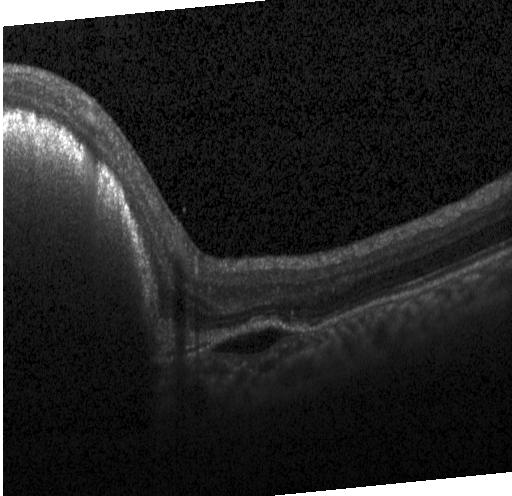
Diagnosis: choroidal neovascularization (CNV).